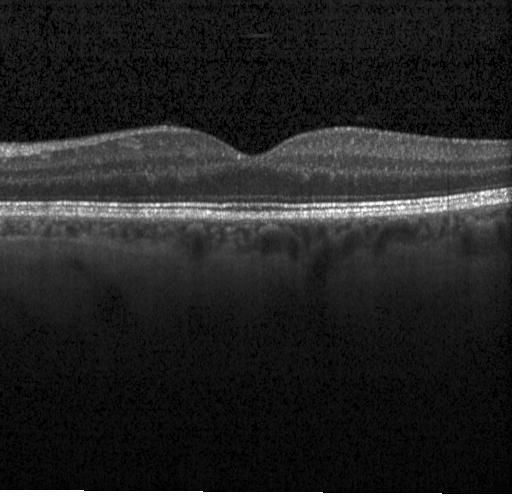

OCT scan showing neither choroidal neovascularization, diabetic macular edema, nor drusen.